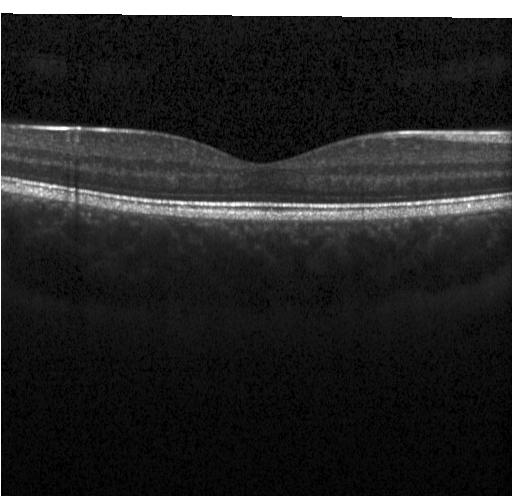

Diagnosis: no choroidal neovascularization, diabetic macular edema, or drusen.